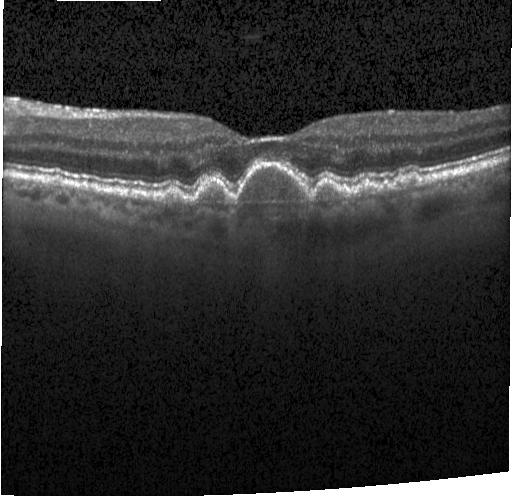

Optical coherence tomography scan
Diagnosis: multiple drusen.